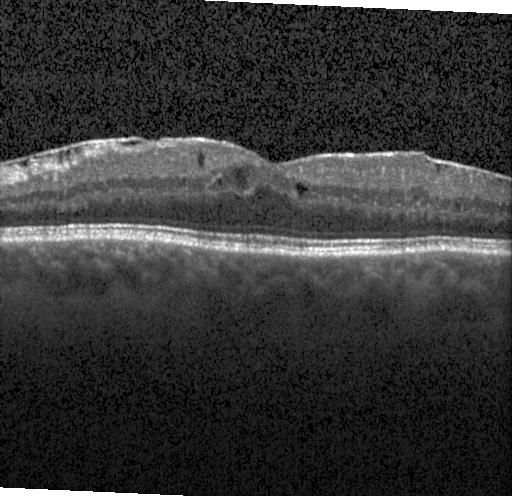 Optical coherence tomography B-scan — This B-scan demonstrates diabetic macular edema (DME).